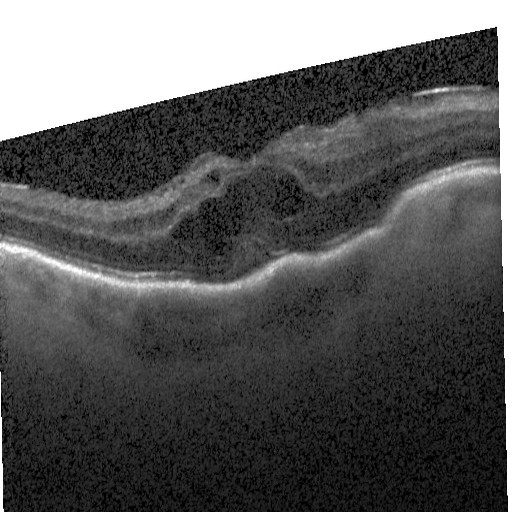
Optical coherence tomography scan · Heidelberg Spectralis. Finding: DME.